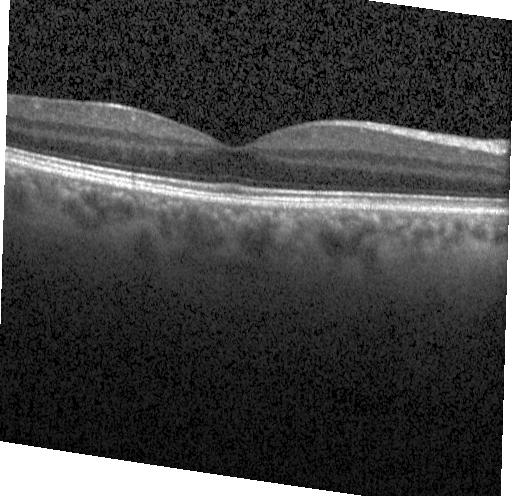 Acquired on a Heidelberg Spectralis, retinal OCT B-scan.
Finding: no evidence of CNV, DME, or drusen.